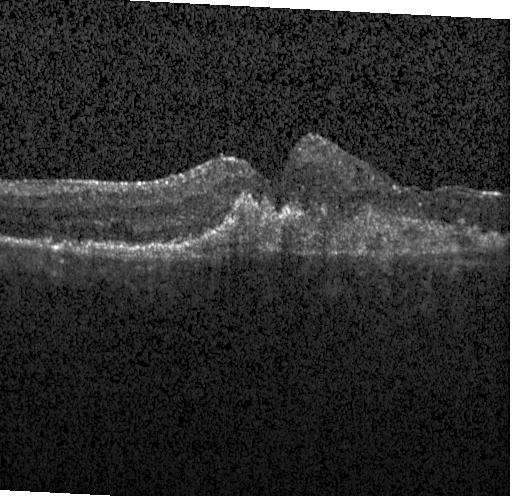 This B-scan demonstrates a choroidal neovascular membrane.